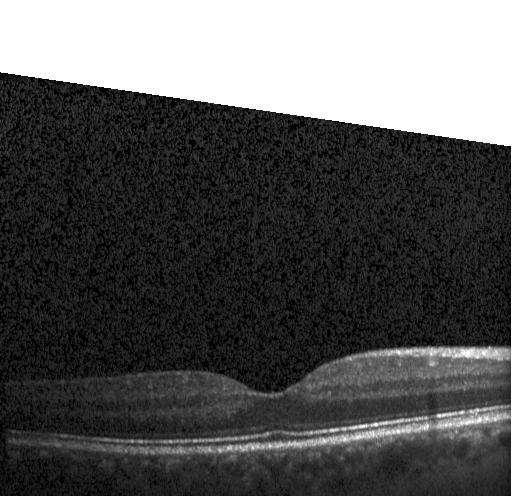

OCT finding: neither choroidal neovascularization, diabetic macular edema, nor drusen.